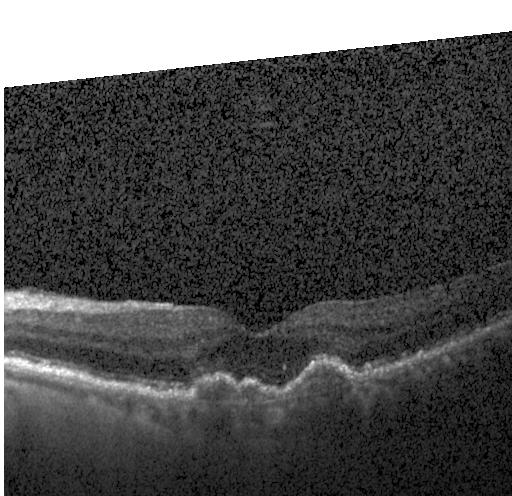
OCT finding: choroidal neovascularization (CNV).